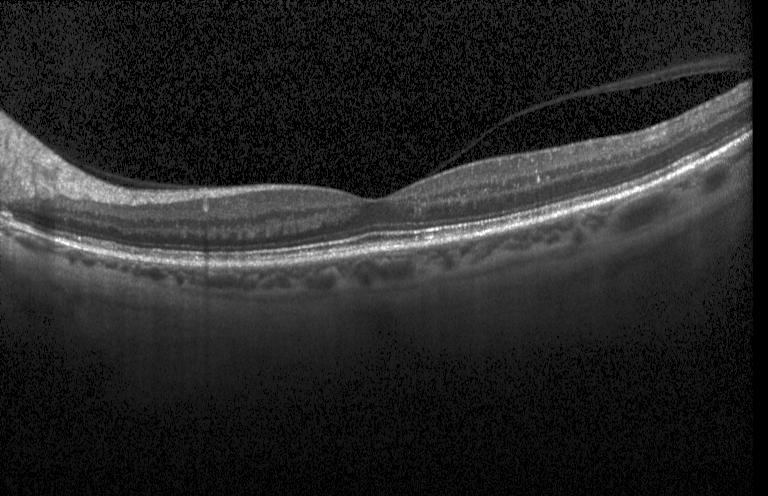 Optical coherence tomography B-scan; horizontal scan through the fovea; acquired on a Heidelberg Spectralis. Diagnosis: no choroidal neovascularization, diabetic macular edema, or drusen.